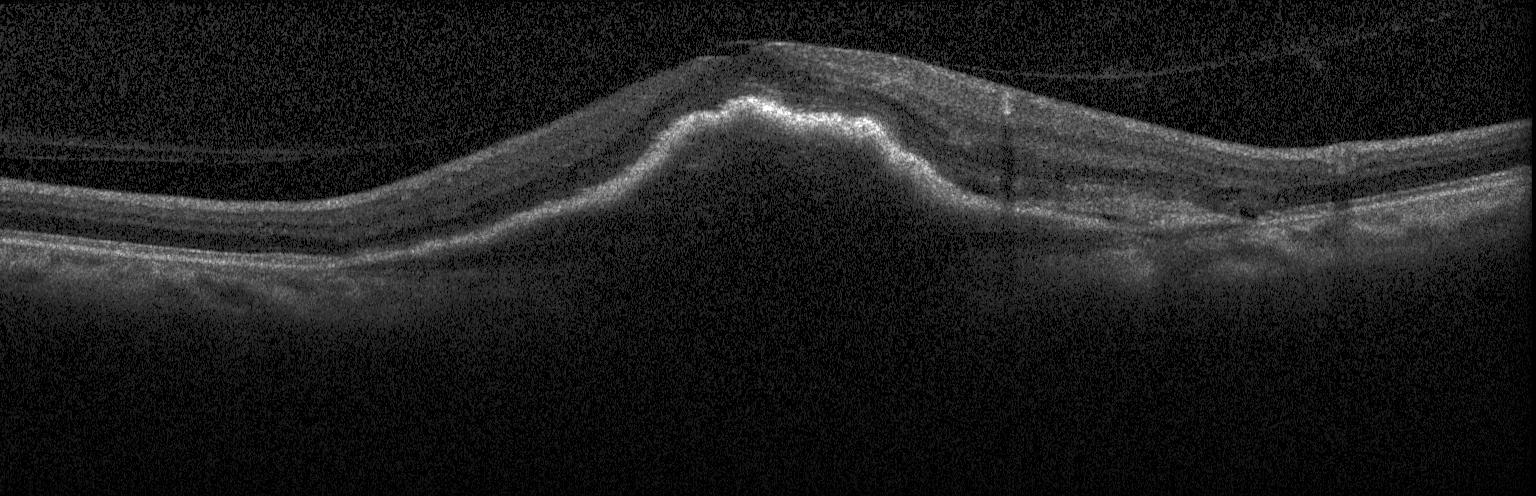

Acquired on a Heidelberg Spectralis, optical coherence tomography scan
Impression: choroidal neovascularization (CNV).